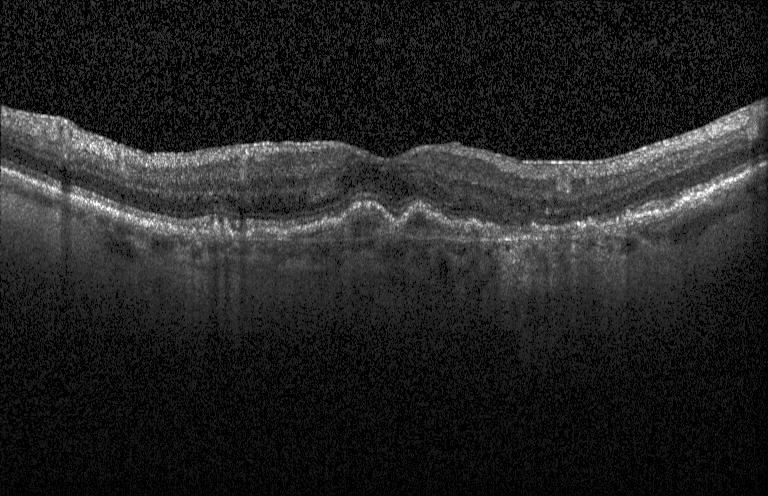 Retinal OCT cross-section.
Finding: CNV.